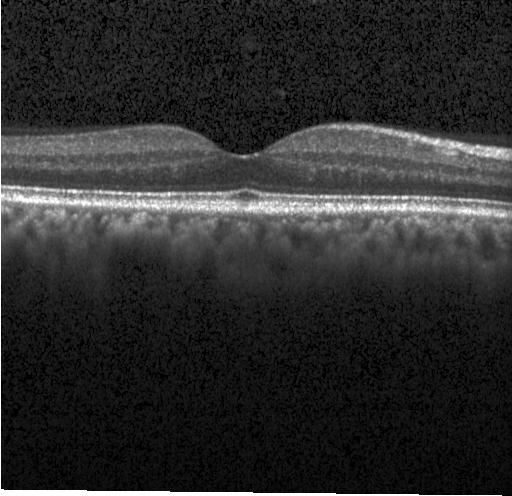 Heidelberg Spectralis. Optical coherence tomography scan. SD-OCT. This B-scan demonstrates no evidence of CNV, DME, or drusen.